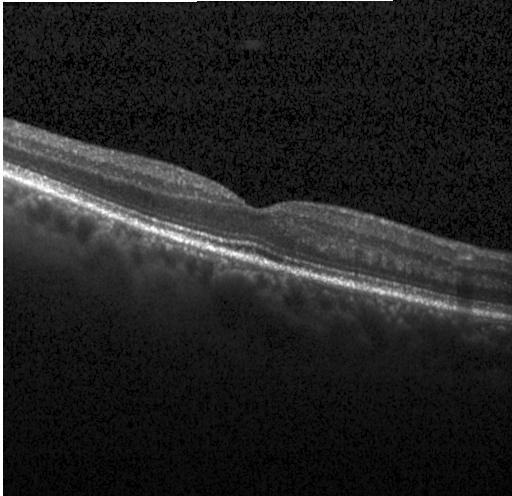 Impression: no choroidal neovascularization, no diabetic macular edema, and no drusen.